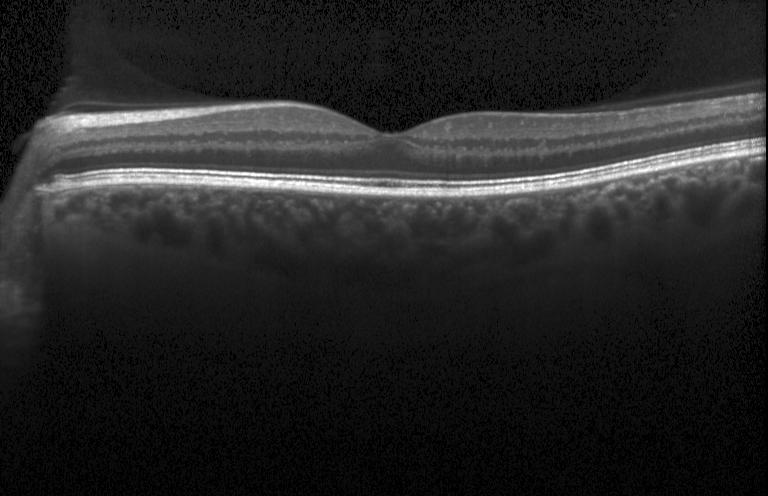

Diagnosis: no evidence of choroidal neovascularization, diabetic macular edema, or drusen.